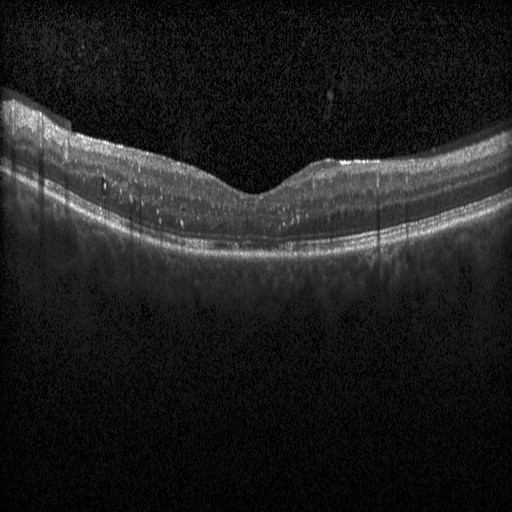
Acquired on a Heidelberg Spectralis. Retinal OCT cross-section. Macular scan
Dx: diabetic macular edema.